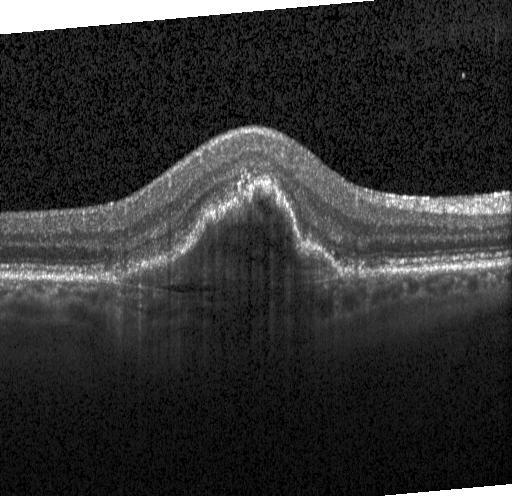
Through the macula, instrument: Heidelberg Spectralis, retinal OCT B-scan
Choroidal neovascularization.